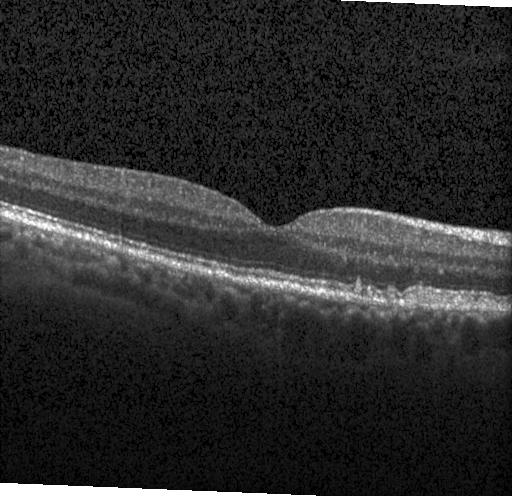
Optical coherence tomography B-scan · Heidelberg Spectralis · SD-OCT · centered on the fovea — The scan shows sub-RPE drusenoid deposits.